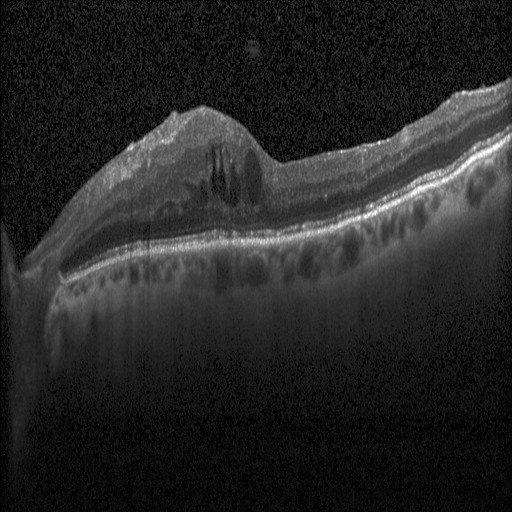 Spectral-domain OCT B-scan: DME.